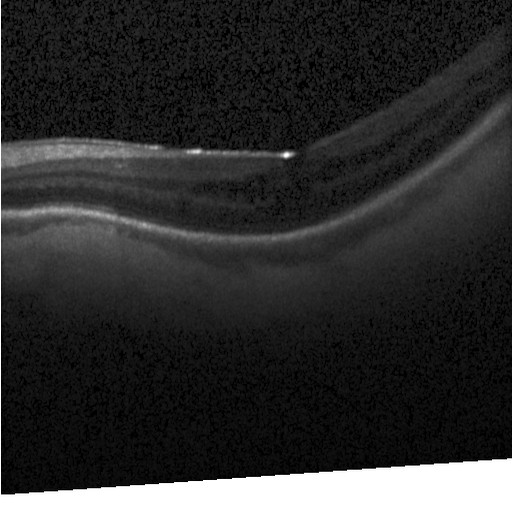
Spectral-domain OCT · instrument: Heidelberg Spectralis · retinal OCT B-scan.
Impression: diabetic macular edema (DME).